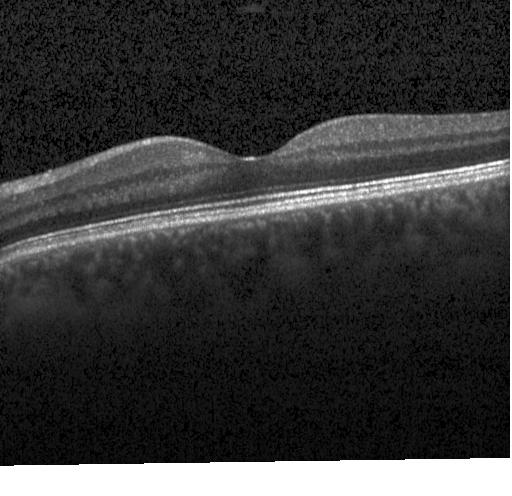 Optical coherence tomography B-scan. Through the macula — Impression: neither CNV, DME, nor drusen.